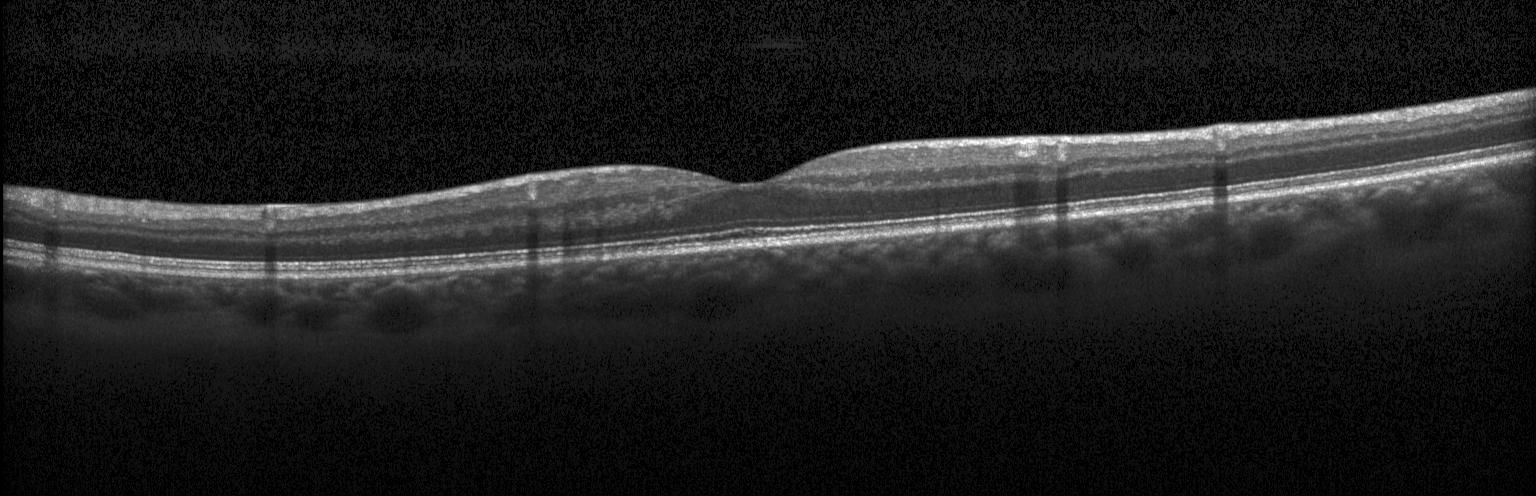
Optical coherence tomography scan.
Assessment: no evidence of CNV, DME, or drusen.